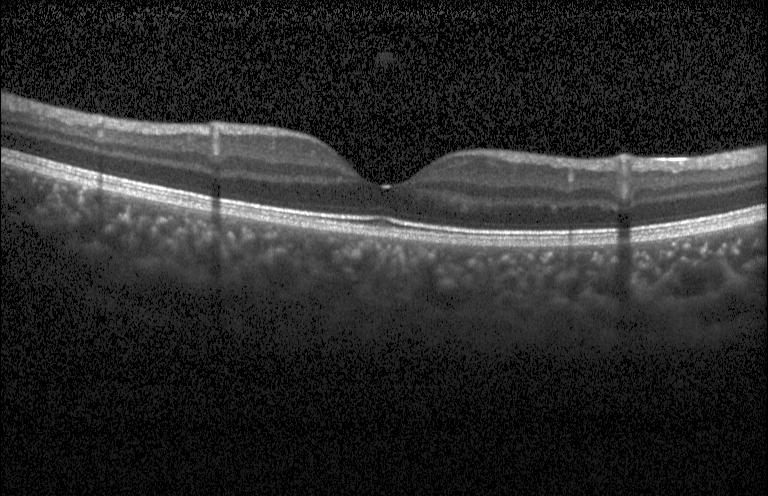

Retinal OCT cross-section.
Dx: no evidence of CNV, DME, or drusen.